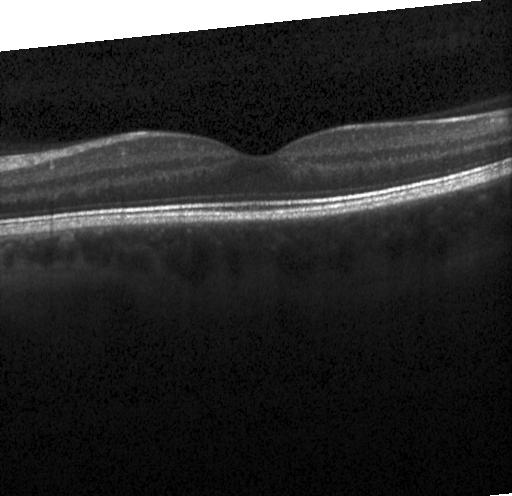

Heidelberg Spectralis; centered on the fovea; optical coherence tomography B-scan; spectral-domain OCT. Finding: no choroidal neovascularization, no diabetic macular edema, and no drusen.